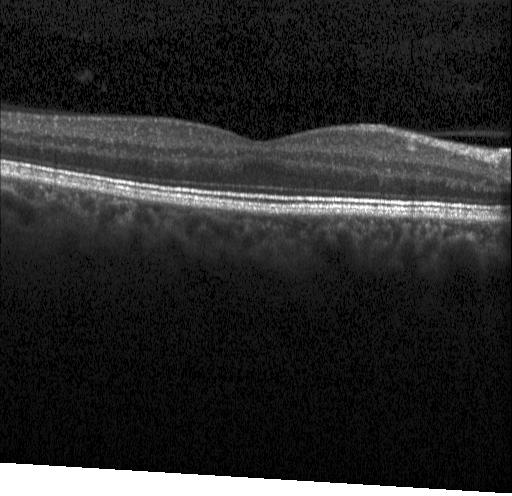

Retinal OCT B-scan; spectral-domain optical coherence tomography; fovea-centered; acquired on a Heidelberg Spectralis.
Diagnosis: neither choroidal neovascularization, diabetic macular edema, nor drusen.